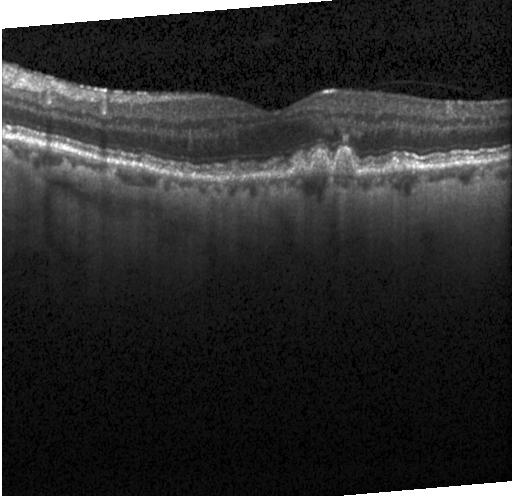

Impression: multiple drusen.